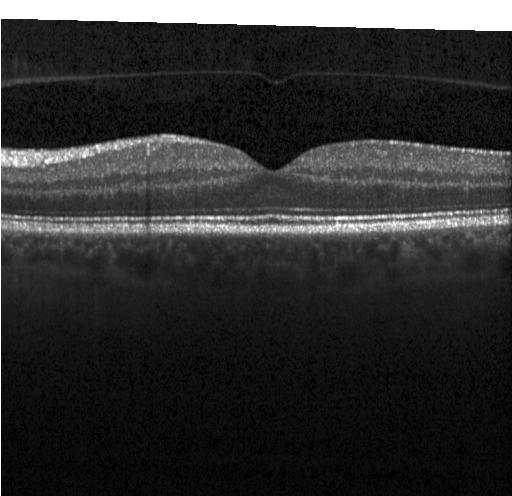 Heidelberg Spectralis OCT system; spectral-domain optical coherence tomography; through the macula; optical coherence tomography B-scan
Finding: no choroidal neovascularization, no diabetic macular edema, and no drusen.